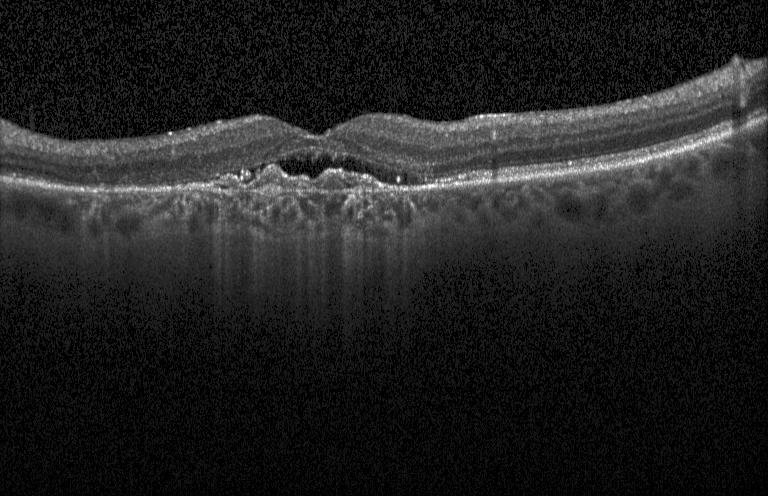

Acquired on a Heidelberg Spectralis · optical coherence tomography scan · spectral-domain optical coherence tomography.
The scan shows a choroidal neovascular membrane.